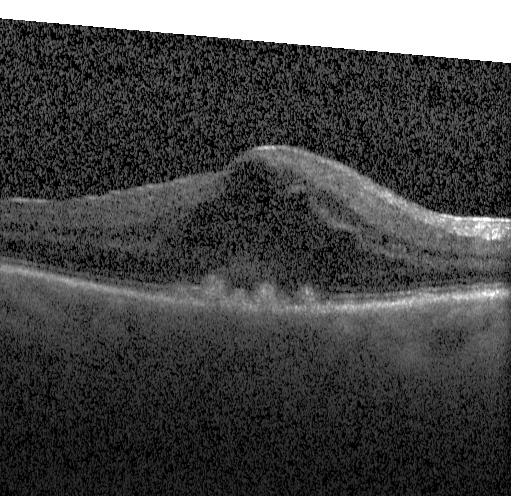 Macular OCT: a choroidal neovascular membrane.